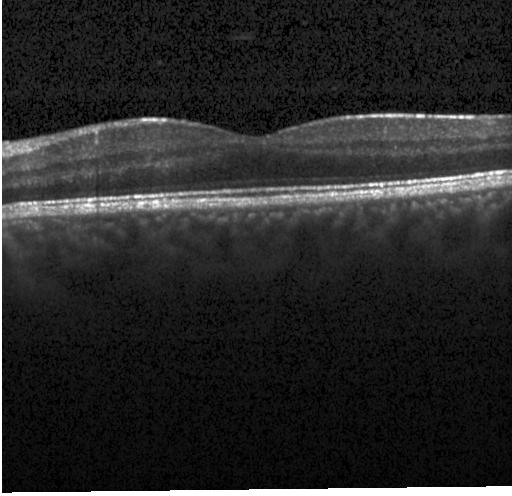

Optical coherence tomography scan. No evidence of choroidal neovascularization, diabetic macular edema, or drusen.